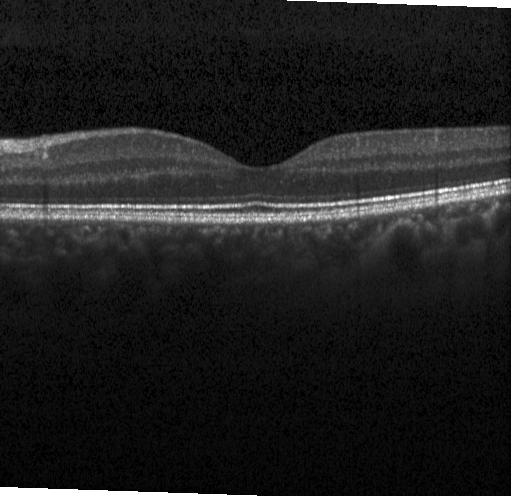
SD-OCT · OCT B-scan.
OCT finding: no choroidal neovascularization, no diabetic macular edema, and no drusen.